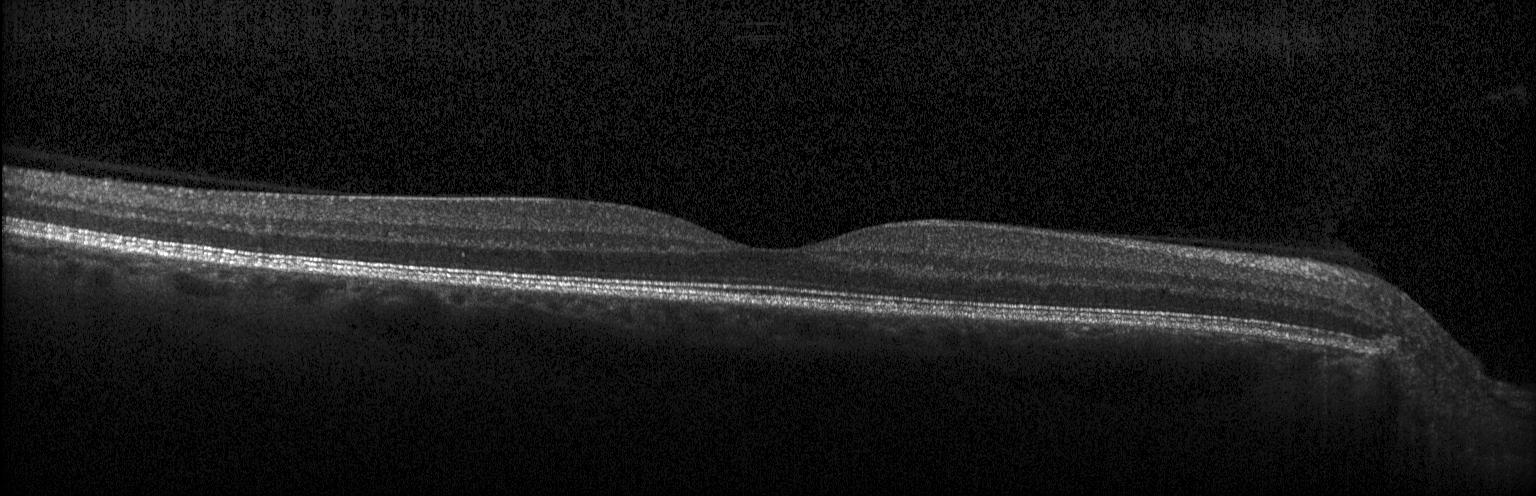 SD-OCT, retinal OCT B-scan, through the macula, Heidelberg Spectralis — Impression: neither choroidal neovascularization, diabetic macular edema, nor drusen.